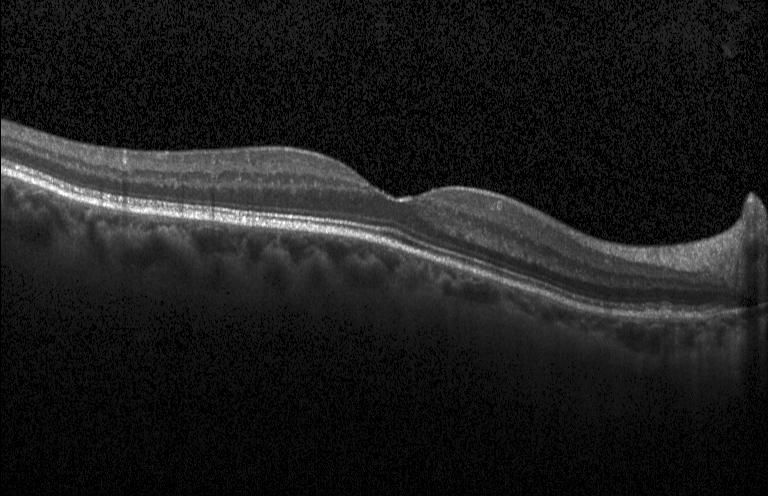 No CNV, no DME, and no drusen.